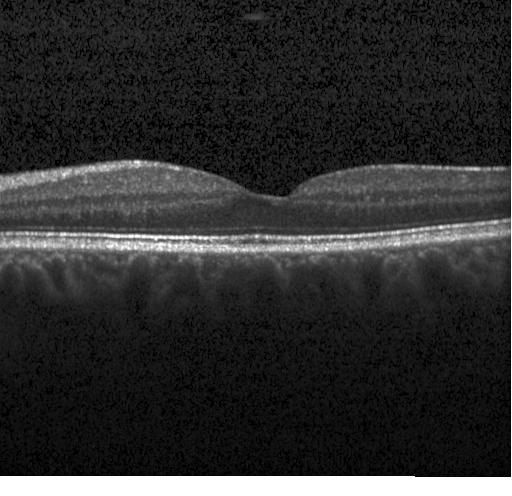 Assessment: neither choroidal neovascularization, diabetic macular edema, nor drusen.